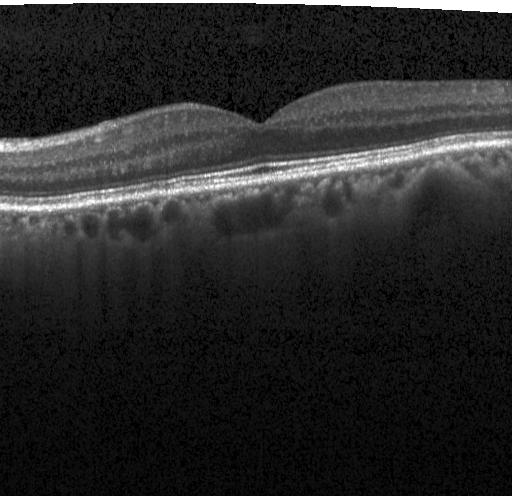 Macular OCT demonstrating no choroidal neovascularization, no diabetic macular edema, and no drusen.